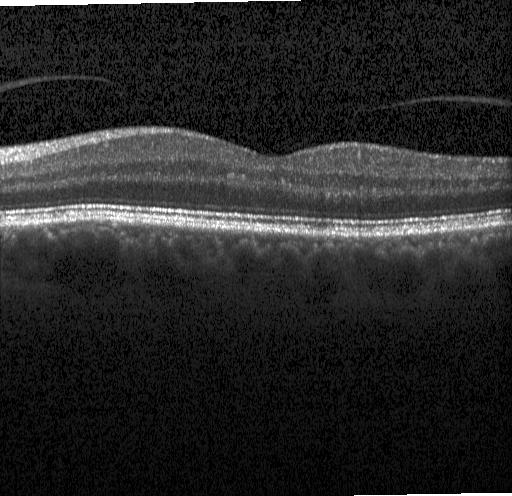
Spectral-domain OCT; Heidelberg Spectralis; optical coherence tomography scan; macular scan
No choroidal neovascularization, diabetic macular edema, or drusen.